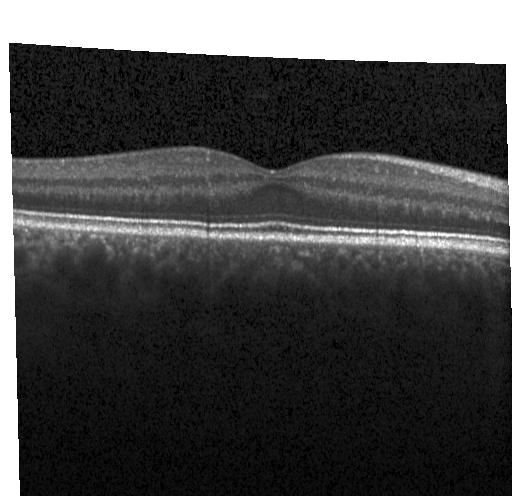 No evidence of CNV, DME, or drusen.